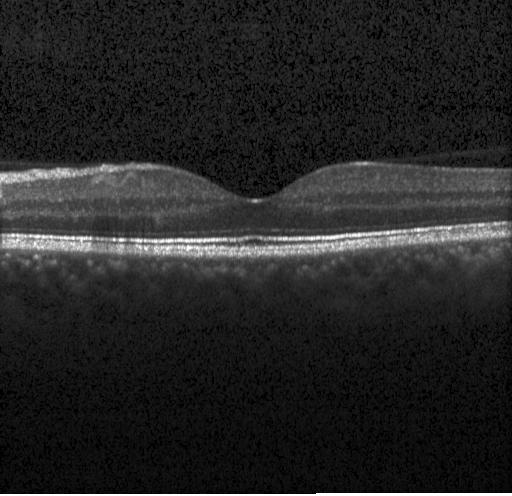

This B-scan demonstrates no choroidal neovascularization, diabetic macular edema, or drusen.